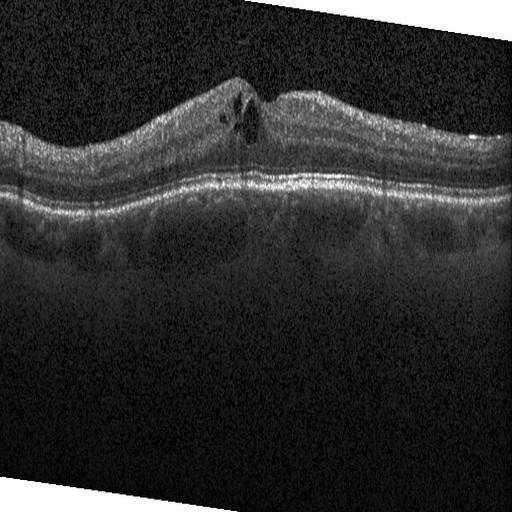
OCT B-scan showing DME.